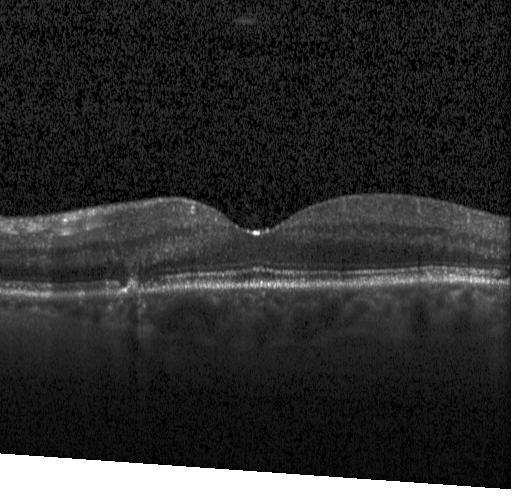

The scan shows multiple drusen.